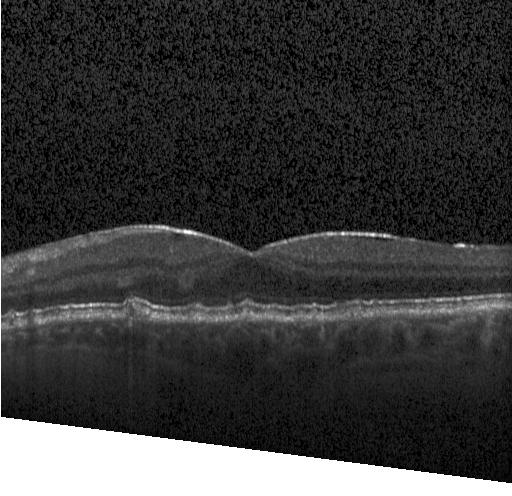 Dx: drusen.